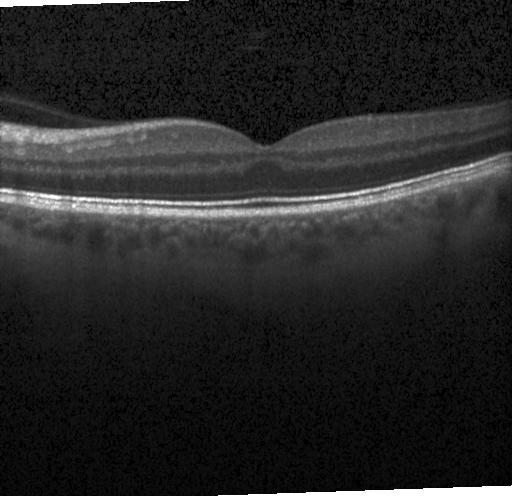
Retinal OCT cross-section
Finding: neither choroidal neovascularization, diabetic macular edema, nor drusen.